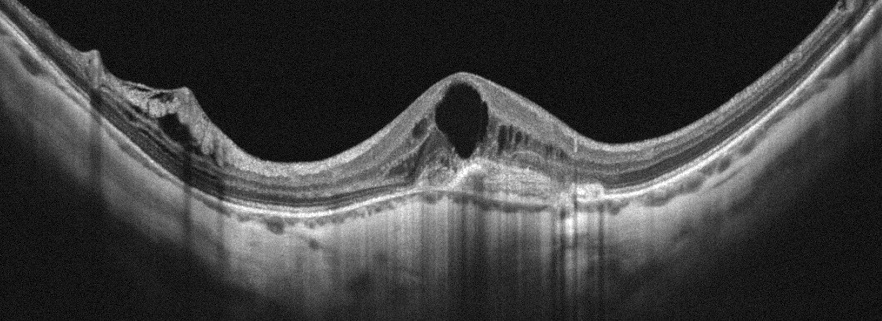
Impression: age-related macular degeneration (AMD).